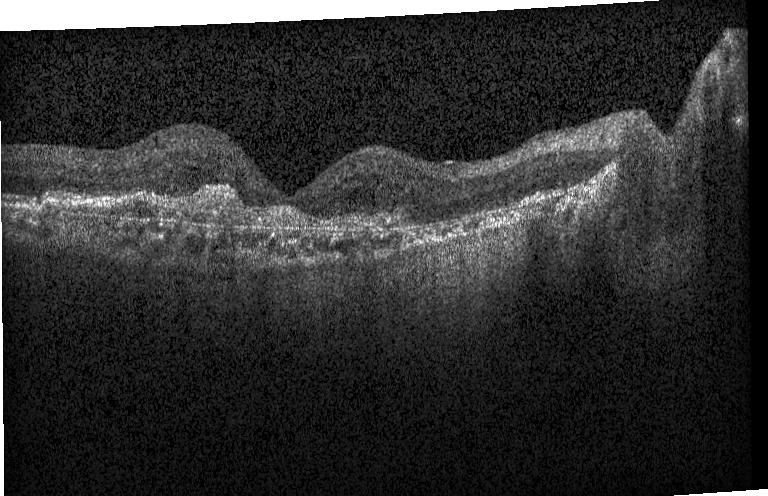

Retinal OCT cross-section
Impression: CNV.